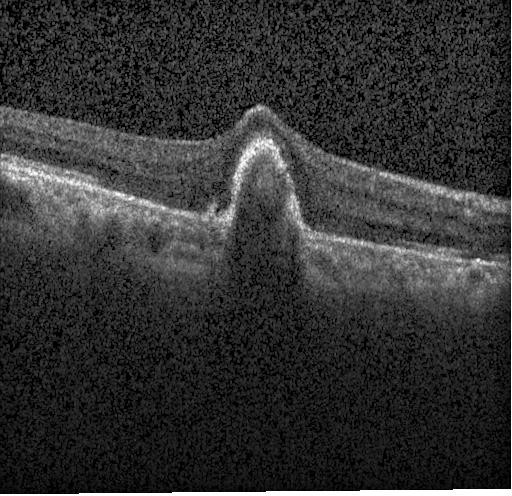
Dx: CNV.